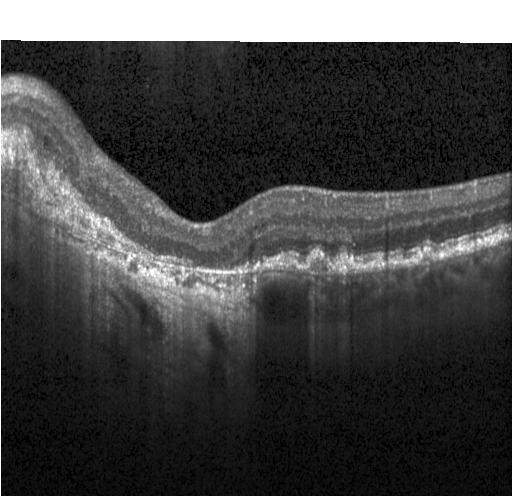
SD-OCT · retinal OCT B-scan
Impression: choroidal neovascularization (CNV).